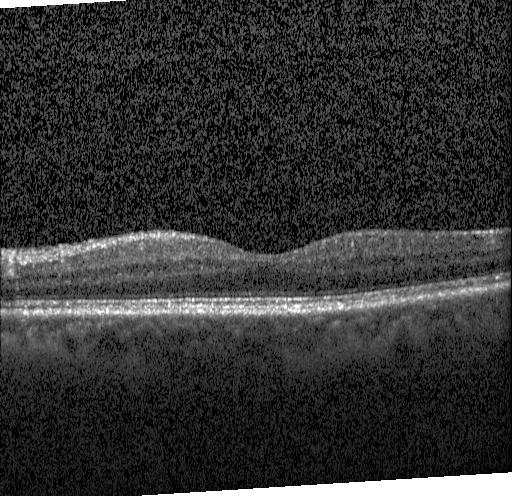

Impression: no CNV, no DME, and no drusen.